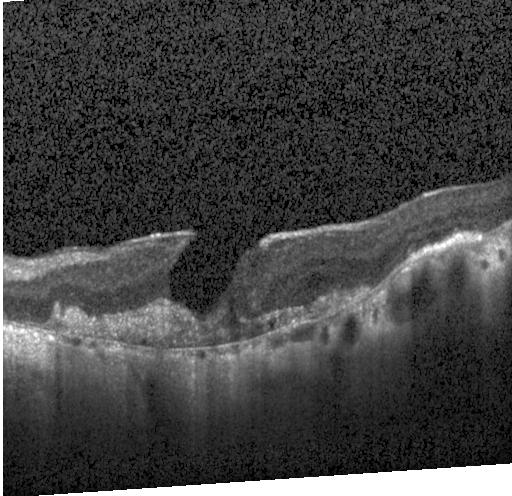
SD-OCT, through the macula, retinal OCT cross-section. Diagnosis: CNV.